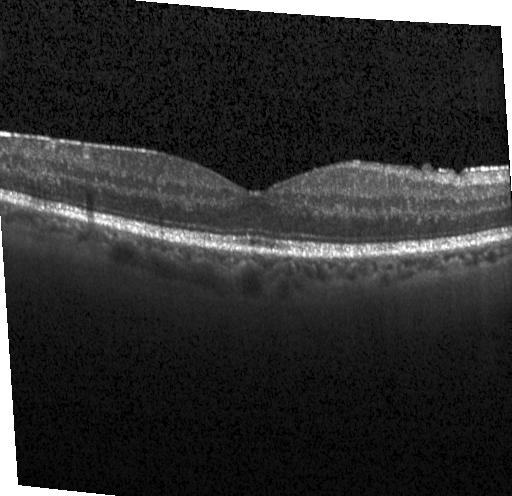 Impression: no evidence of choroidal neovascularization, diabetic macular edema, or drusen.